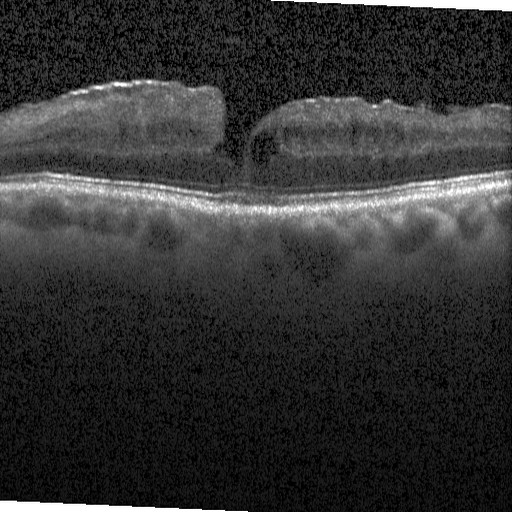
OCT B-scan; spectral-domain optical coherence tomography; acquired on a Heidelberg Spectralis; centered on the fovea — Macular OCT: diabetic macular edema (DME).